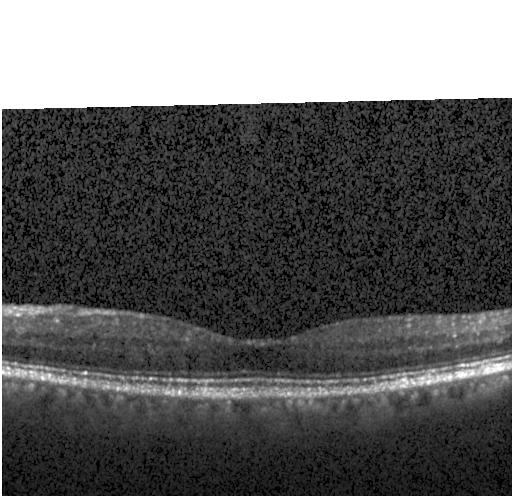
Assessment: no evidence of choroidal neovascularization, diabetic macular edema, or drusen.